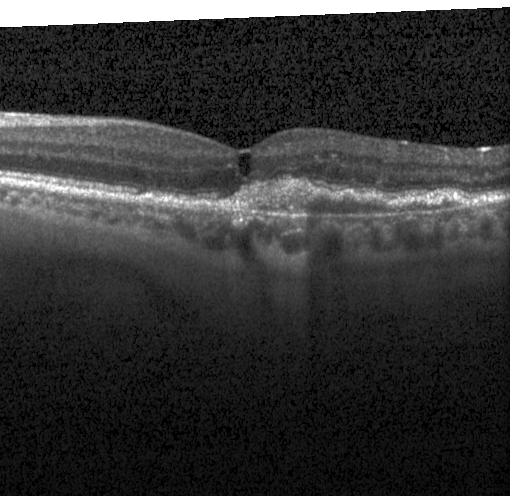 OCT scan showing a choroidal neovascular membrane.